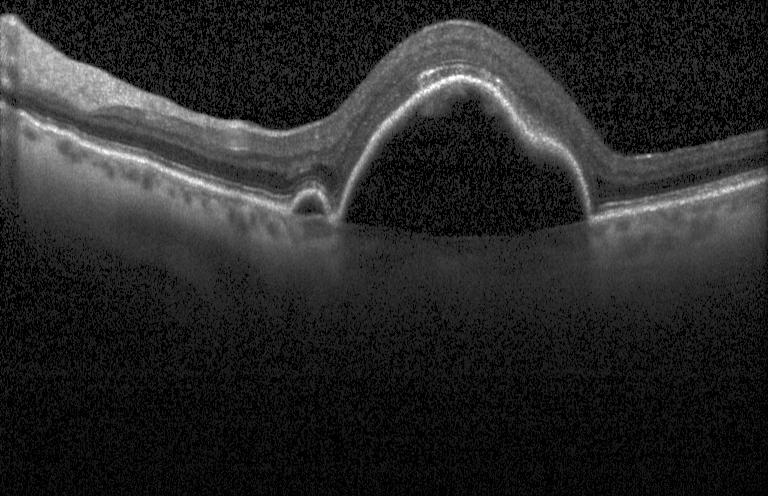

Macular scan · acquired on a Heidelberg Spectralis · retinal OCT B-scan · SD-OCT.
Finding: choroidal neovascularization (CNV).